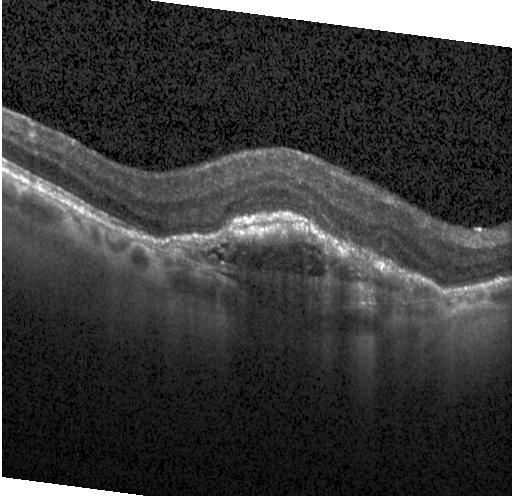
OCT finding: a choroidal neovascular membrane.